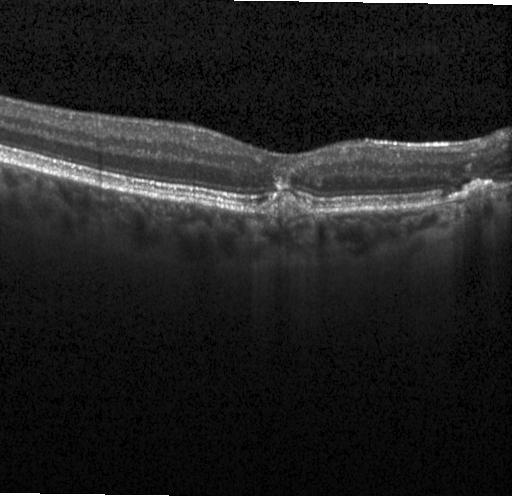 Acquired on a Heidelberg Spectralis · through the macula · spectral-domain optical coherence tomography · retinal OCT cross-section — The scan shows sub-RPE drusenoid deposits.